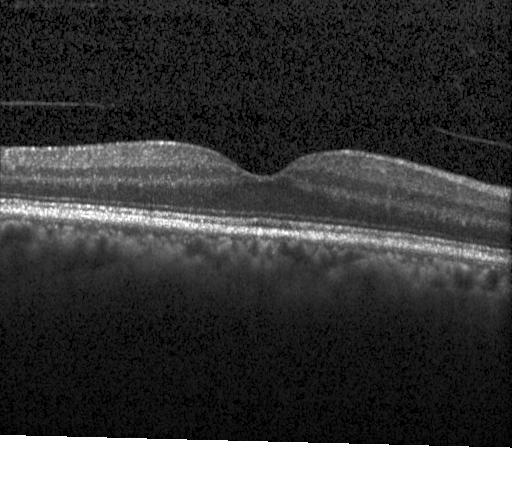

Finding: neither choroidal neovascularization, diabetic macular edema, nor drusen.